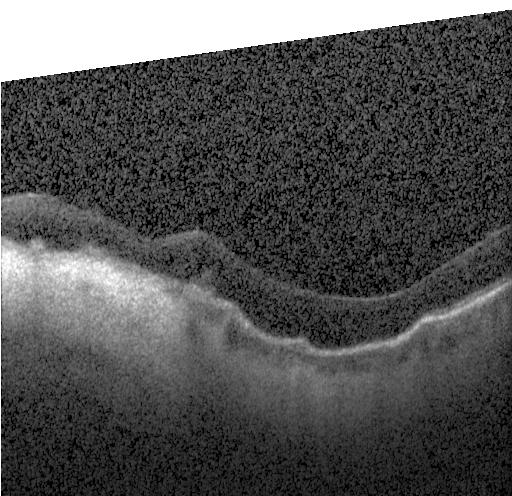
Retinal OCT cross-section showing choroidal neovascularization.